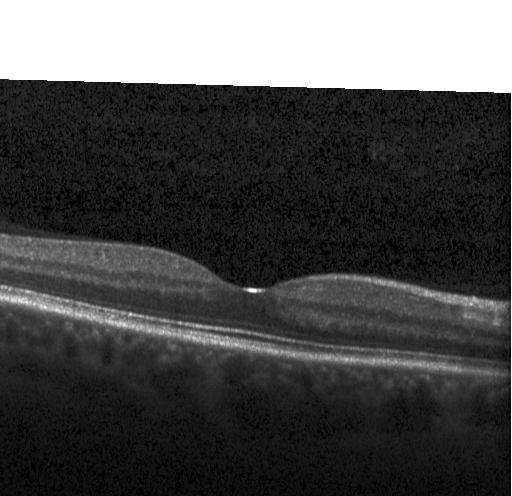

Optical coherence tomography scan.
Neither choroidal neovascularization, diabetic macular edema, nor drusen.